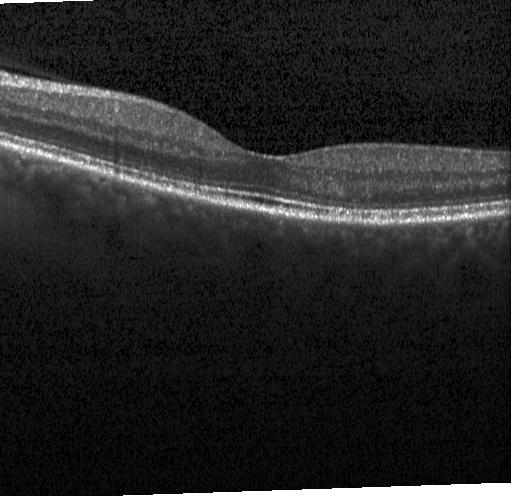
Finding: no evidence of choroidal neovascularization, diabetic macular edema, or drusen.